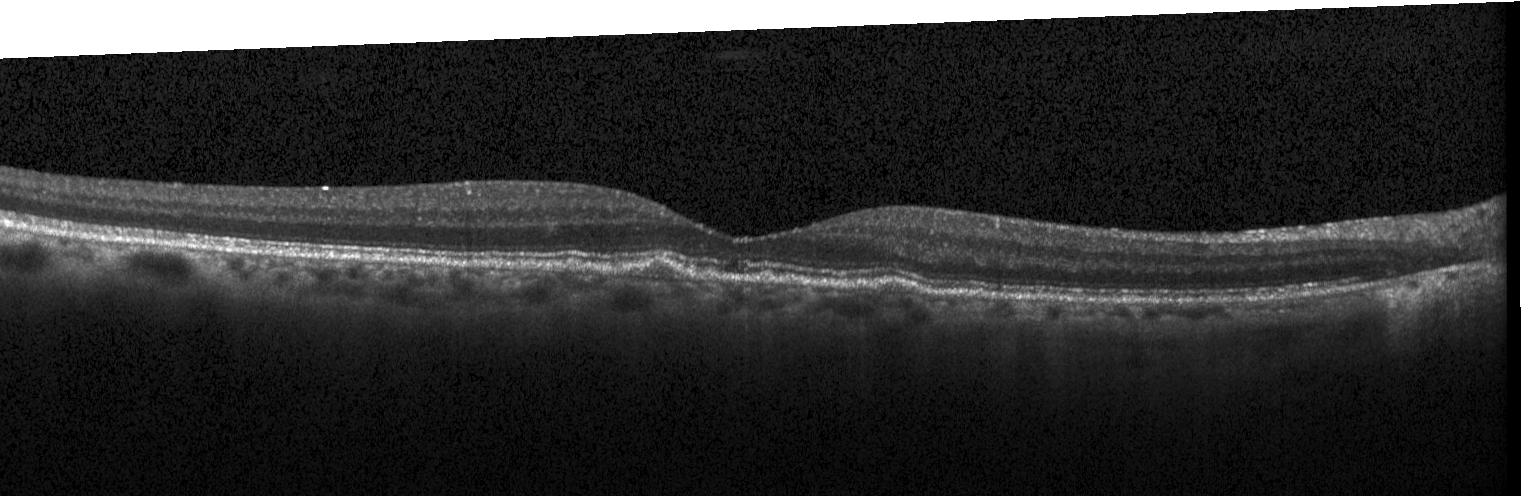
OCT B-scan showing sub-RPE drusenoid deposits.